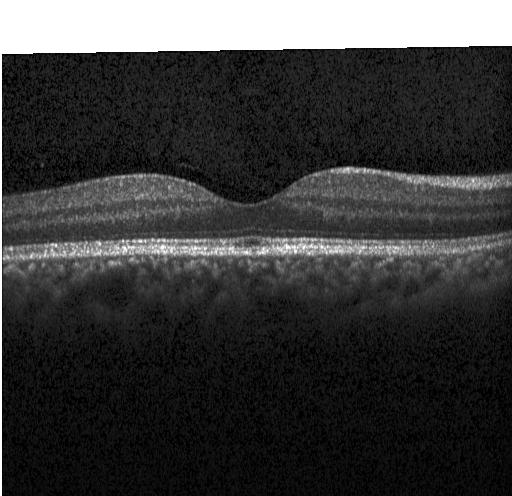 Retinal OCT cross-section showing no evidence of choroidal neovascularization, diabetic macular edema, or drusen.